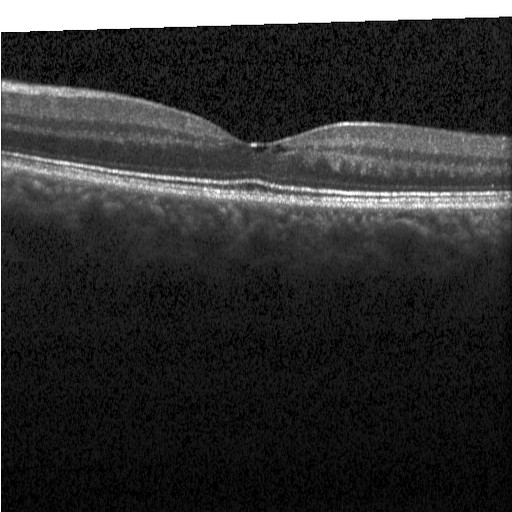
Retinal OCT B-scan. Instrument: Heidelberg Spectralis. Horizontal scan through the fovea.
This B-scan demonstrates DME.